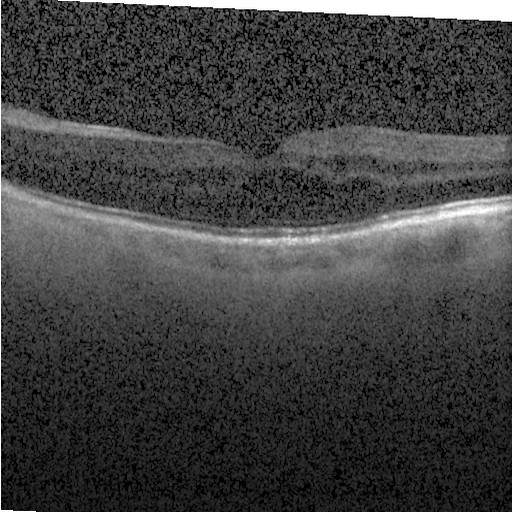

Optical coherence tomography B-scan
OCT finding: DME.